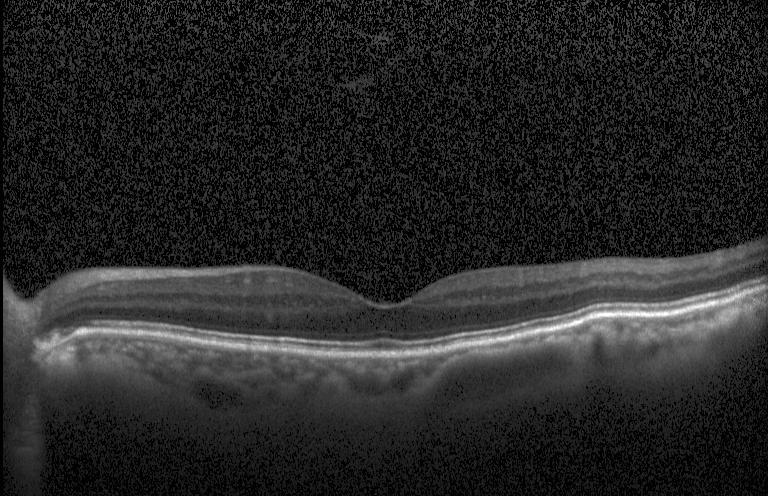
OCT line scan.
This B-scan demonstrates no CNV, no DME, and no drusen.